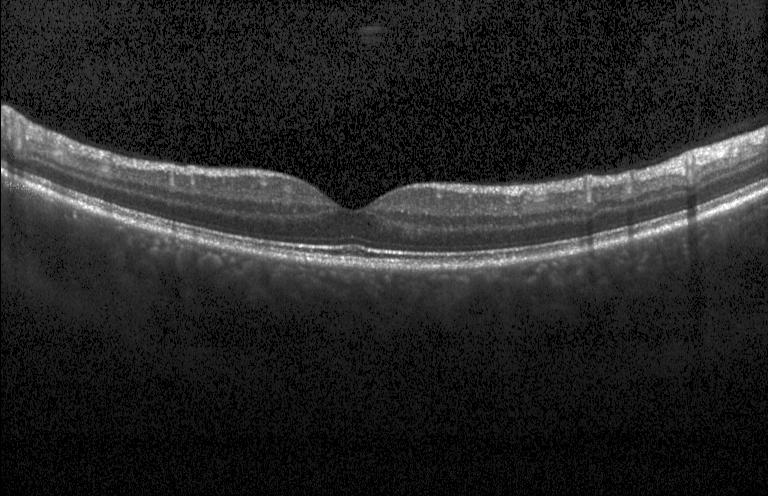

Finding: no CNV, DME, or drusen.